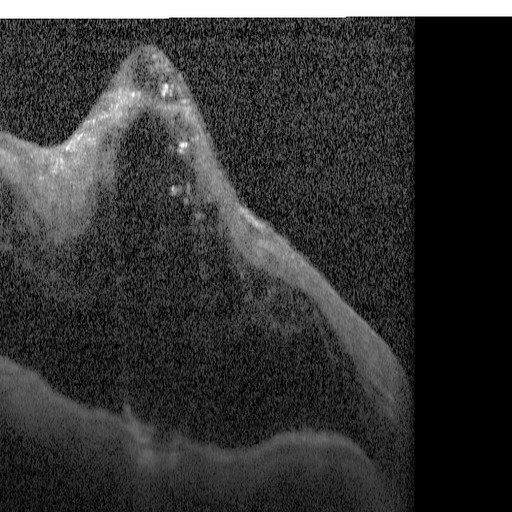 This B-scan demonstrates diabetic macular edema.